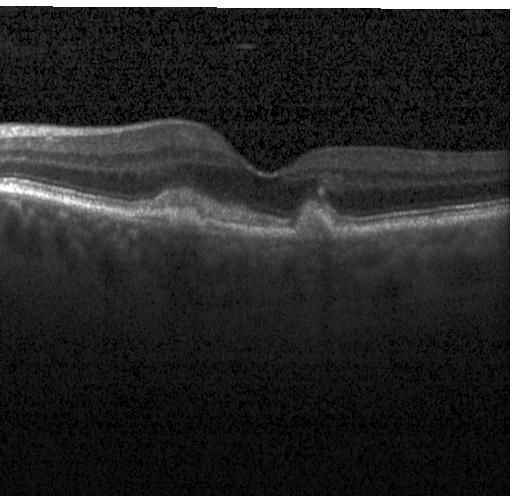
OCT B-scan · Heidelberg Spectralis OCT system · spectral-domain optical coherence tomography. Diagnosis: choroidal neovascularization.